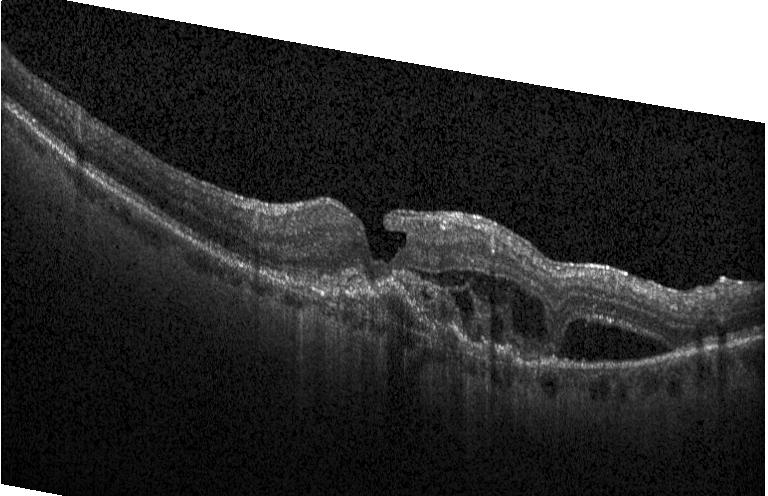 OCT scan showing choroidal neovascularization.